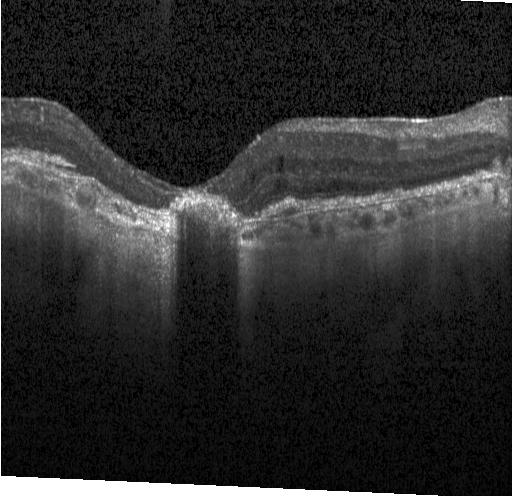 OCT scan showing a choroidal neovascular membrane.